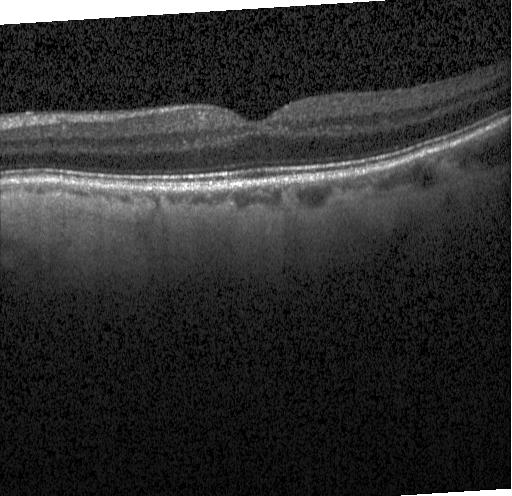
SD-OCT, retinal OCT cross-section. Assessment: no evidence of CNV, DME, or drusen.